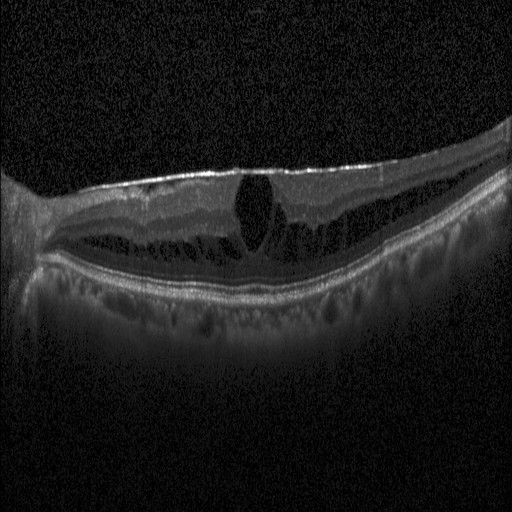

SD-OCT; Heidelberg Spectralis OCT system; fovea-centered; retinal OCT cross-section. Diagnosis: DME.